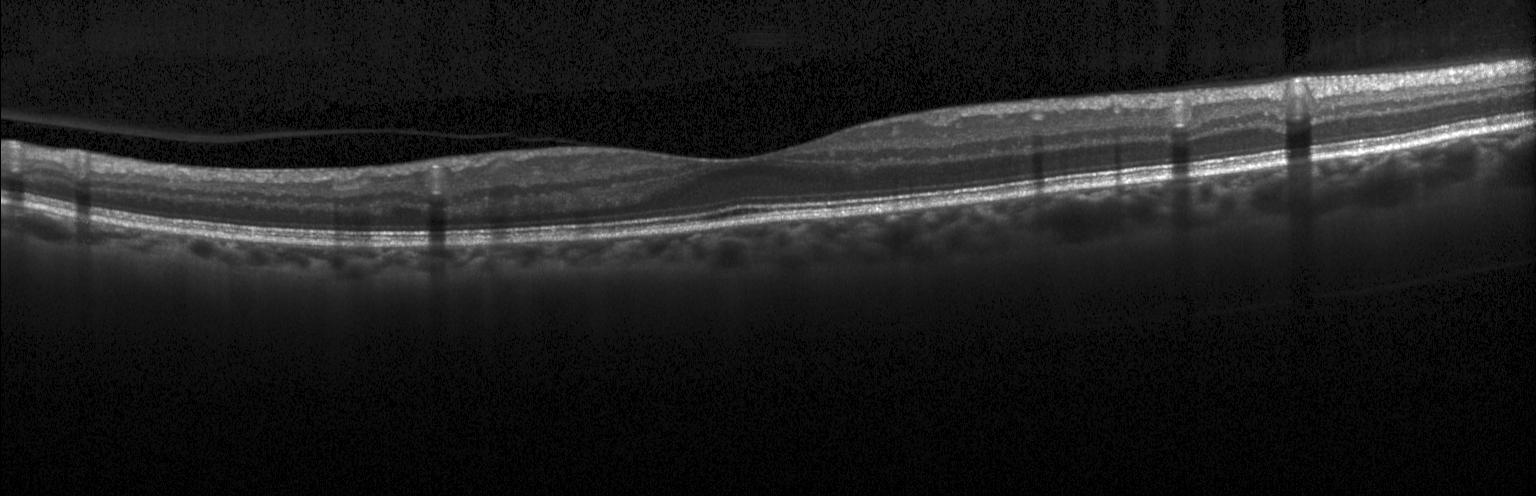

Spectral-domain OCT; fovea-centered; instrument: Heidelberg Spectralis; OCT B-scan. This B-scan demonstrates no evidence of choroidal neovascularization, diabetic macular edema, or drusen.